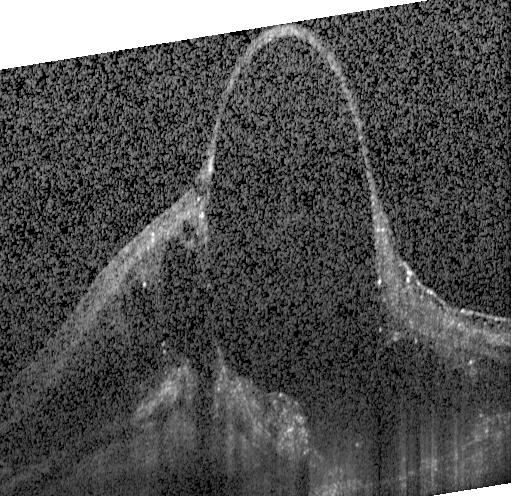
Through the macula; optical coherence tomography B-scan; Heidelberg Spectralis OCT system
Diagnosis: a choroidal neovascular membrane.